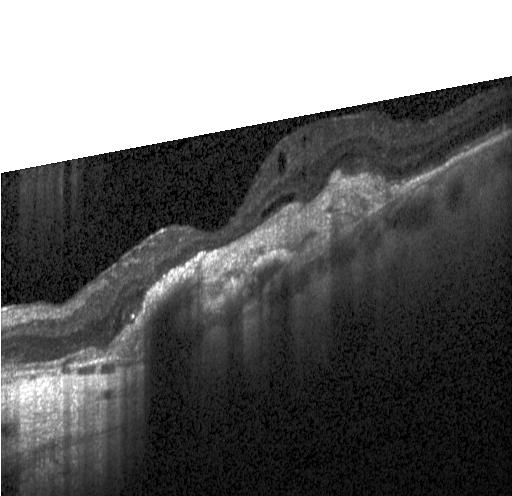 OCT finding: a choroidal neovascular membrane.